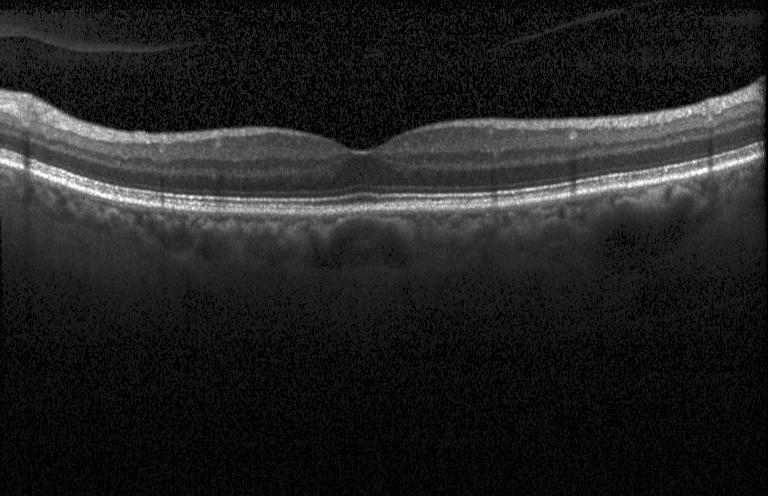
Optical coherence tomography scan.
Impression: no choroidal neovascularization, diabetic macular edema, or drusen.